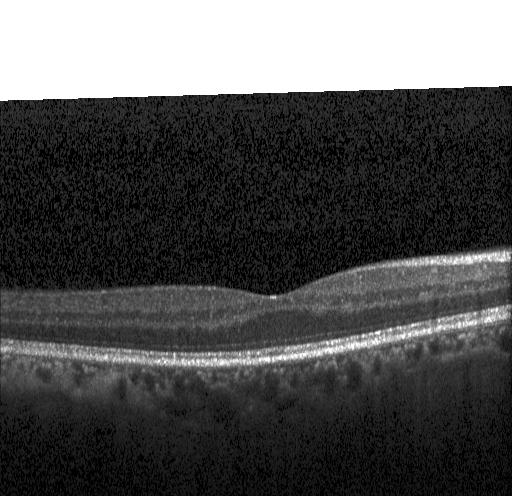
Optical coherence tomography B-scan · through the macula.
This B-scan demonstrates no choroidal neovascularization, diabetic macular edema, or drusen.